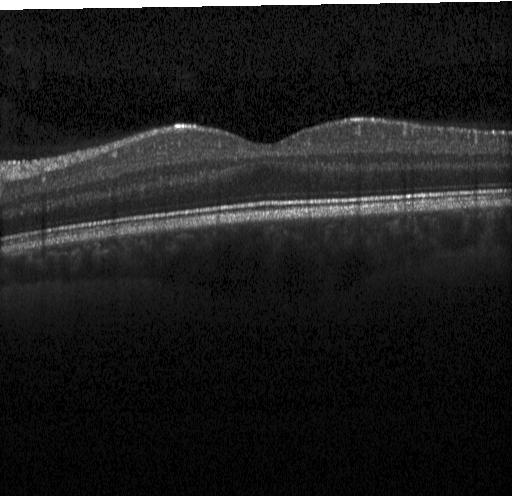

Heidelberg Spectralis OCT system · spectral-domain OCT · optical coherence tomography B-scan
Finding: neither CNV, DME, nor drusen.